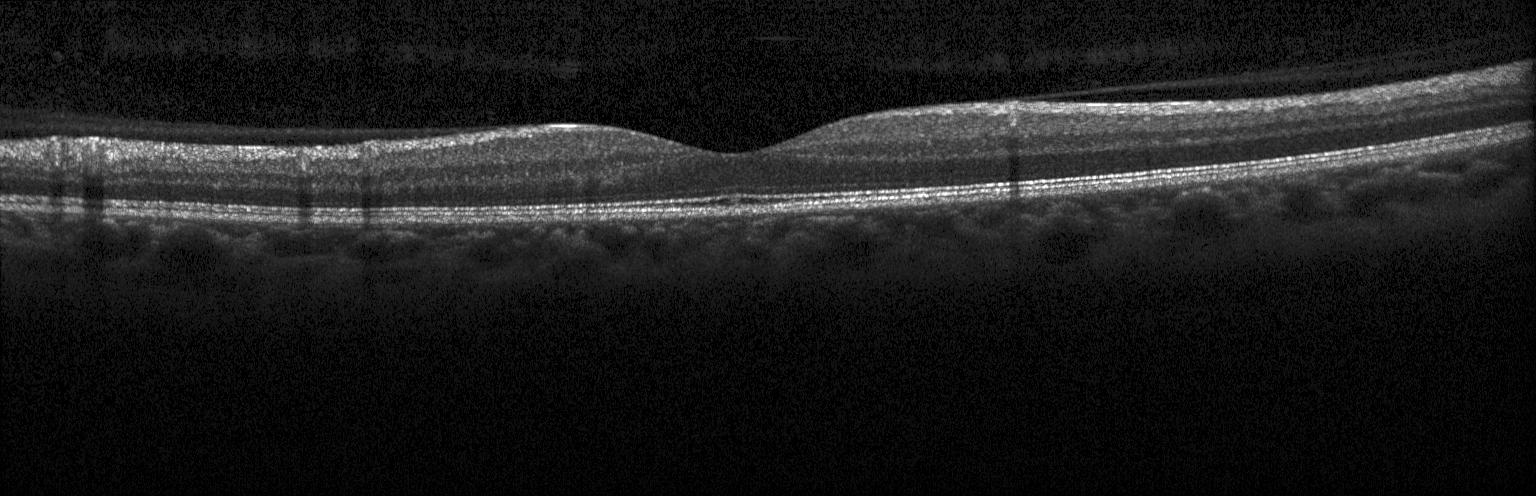
OCT line scan
OCT finding: no choroidal neovascularization, no diabetic macular edema, and no drusen.